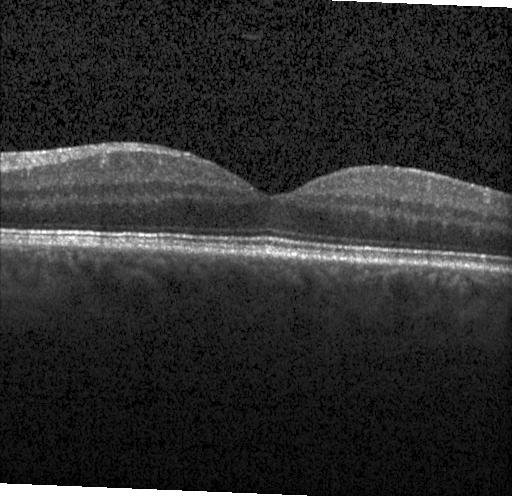

Diagnosis: neither CNV, DME, nor drusen.